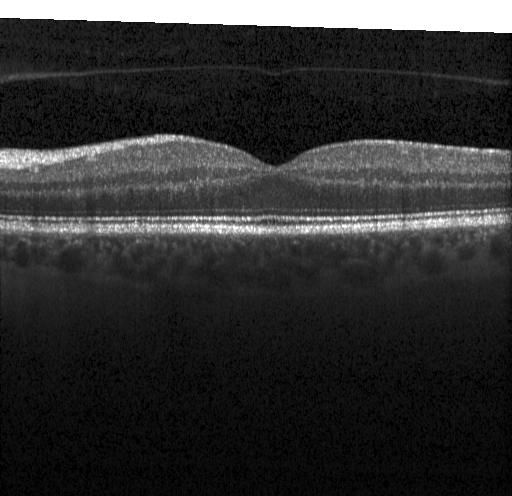
OCT line scan, spectral-domain optical coherence tomography, horizontal scan through the fovea, Heidelberg Spectralis OCT system. Assessment: neither choroidal neovascularization, diabetic macular edema, nor drusen.